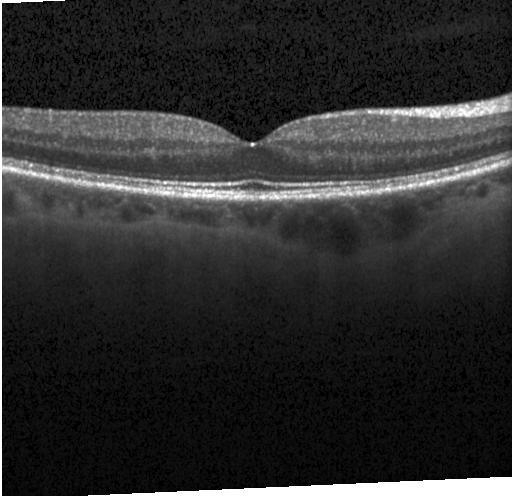

OCT B-scan. Dx: no choroidal neovascularization, diabetic macular edema, or drusen.